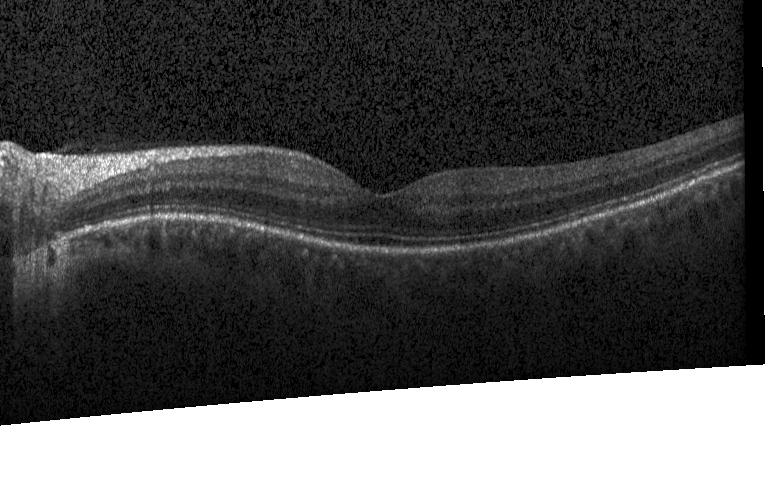
Horizontal scan through the fovea · acquired on a Heidelberg Spectralis · optical coherence tomography scan — Impression: no evidence of choroidal neovascularization, diabetic macular edema, or drusen.